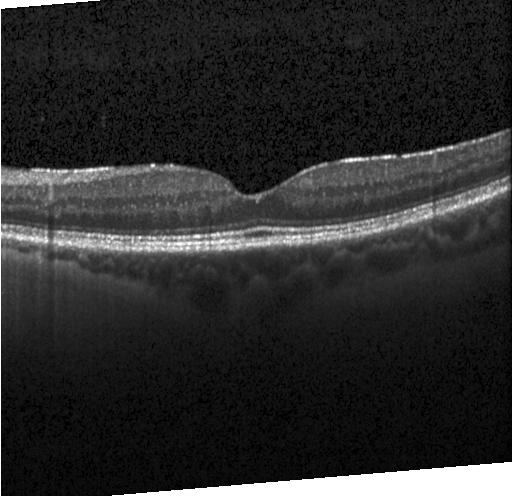 Spectral-domain OCT B-scan: no CNV, no DME, and no drusen.